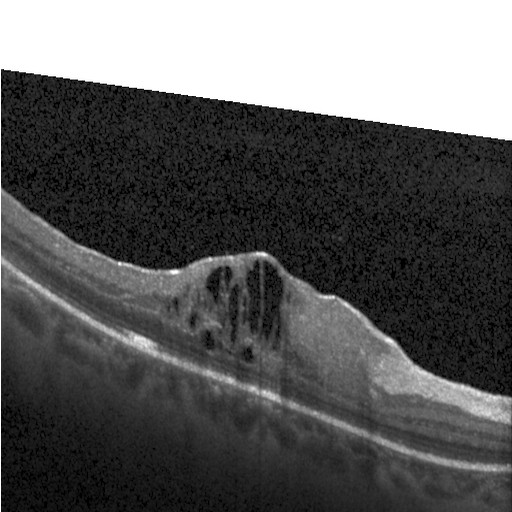

Optical coherence tomography scan.
Diagnosis: DME.